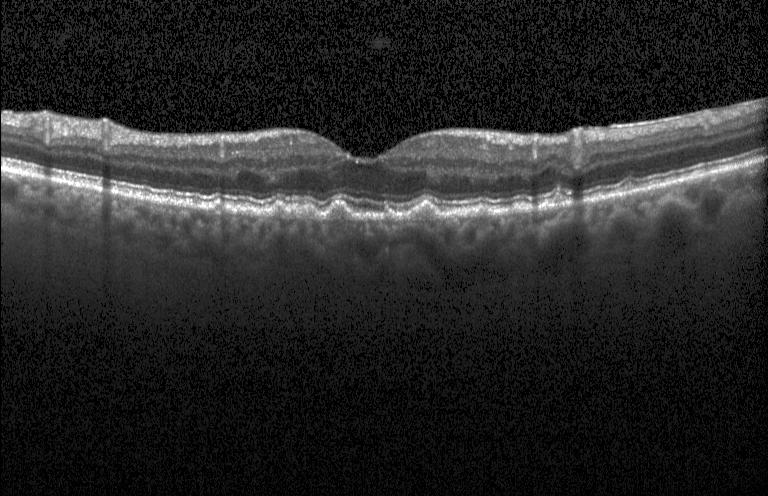

Optical coherence tomography B-scan. Diagnosis: drusen.